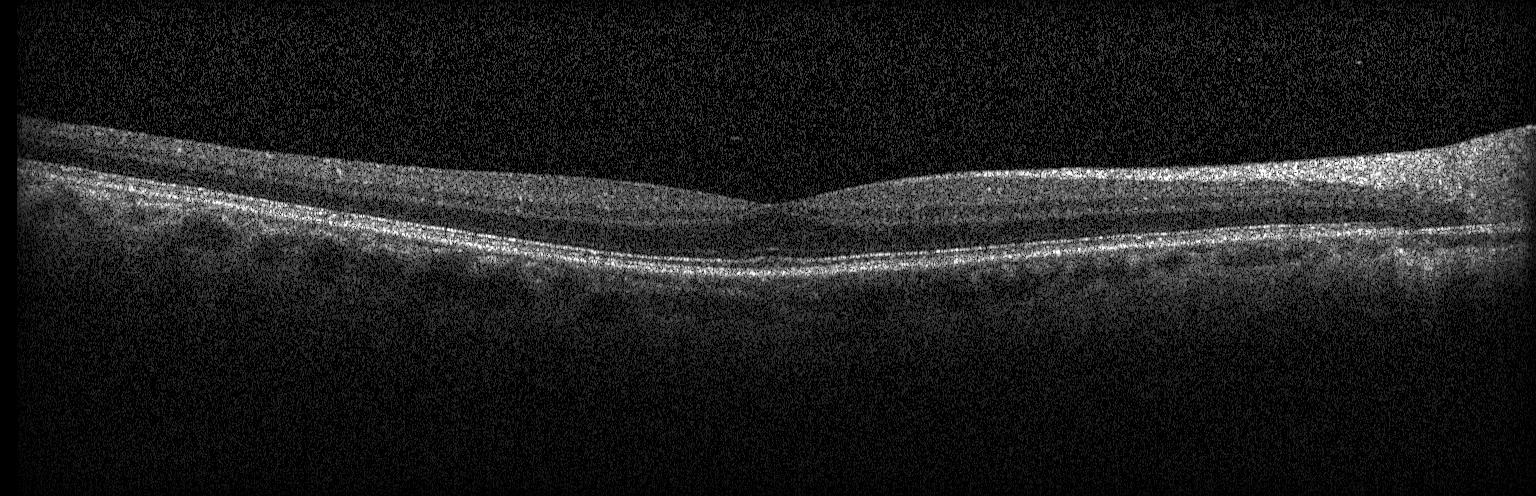 Macular OCT: no CNV, DME, or drusen.